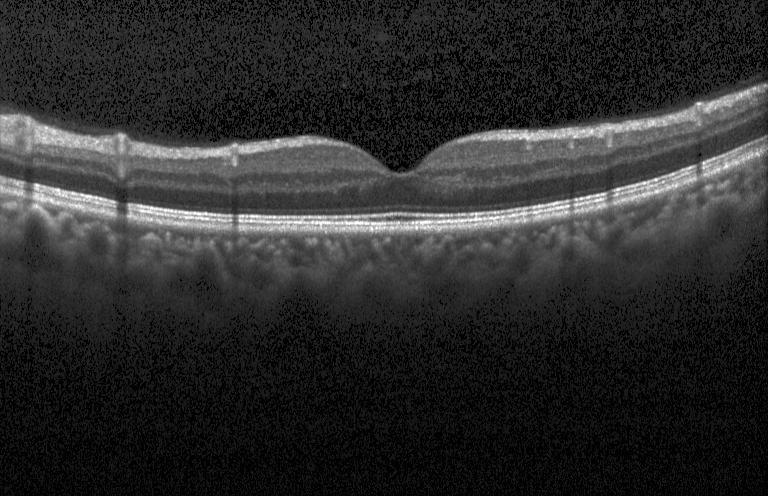

Spectral-domain OCT, optical coherence tomography B-scan.
Impression: neither choroidal neovascularization, diabetic macular edema, nor drusen.